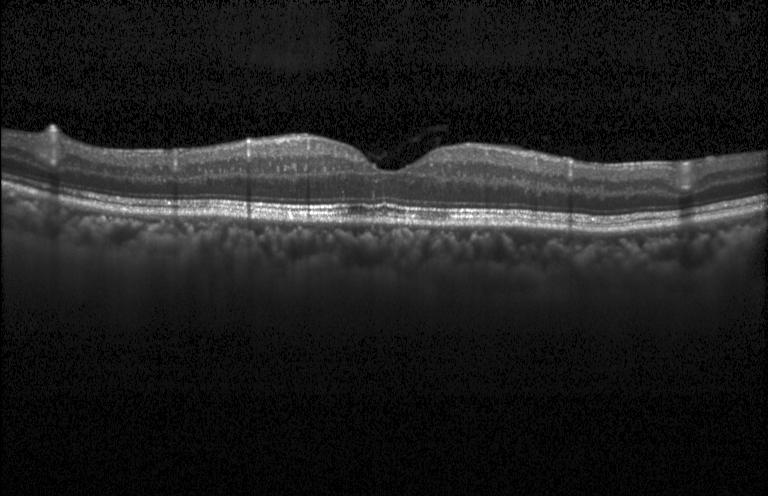

Retinal OCT cross-section · macular scan
No evidence of choroidal neovascularization, diabetic macular edema, or drusen.